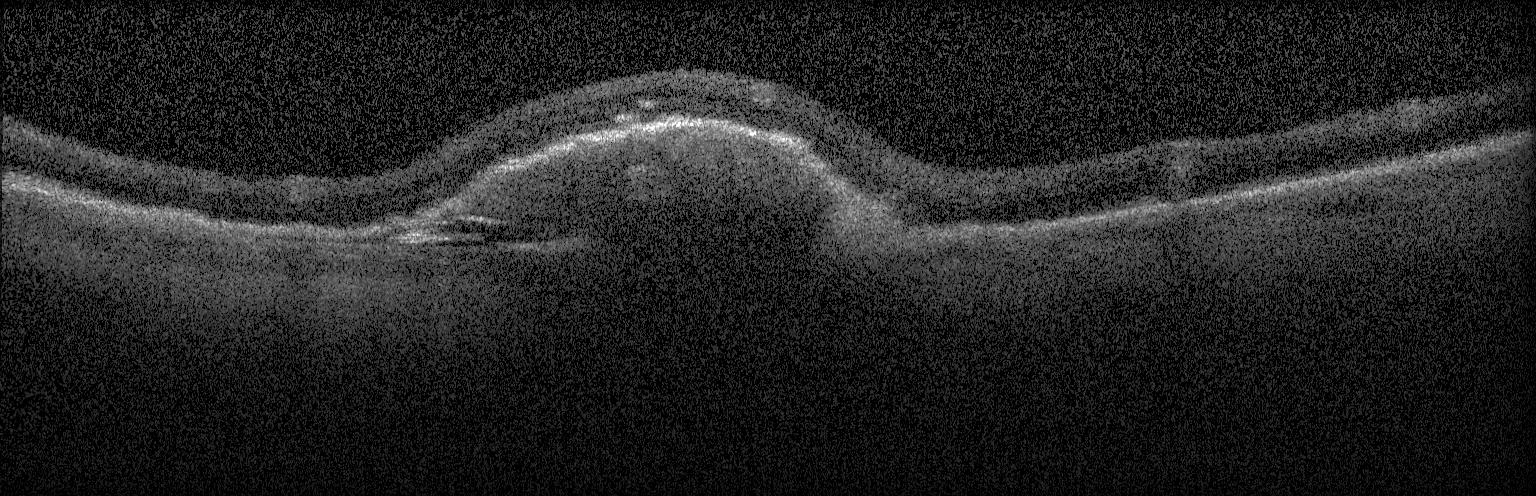

Optical coherence tomography B-scan, instrument: Heidelberg Spectralis, spectral-domain OCT — Finding: a choroidal neovascular membrane.